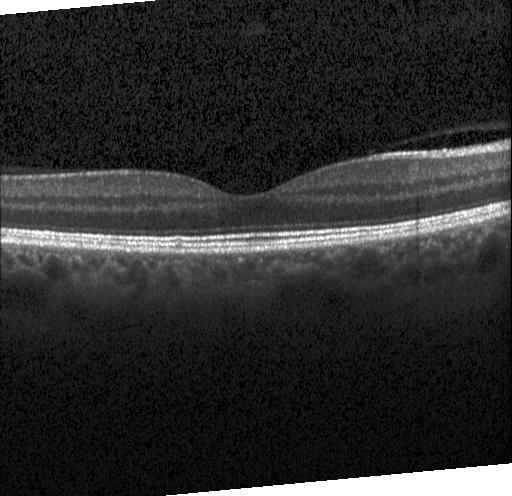 Optical coherence tomography B-scan
Dx: neither choroidal neovascularization, diabetic macular edema, nor drusen.